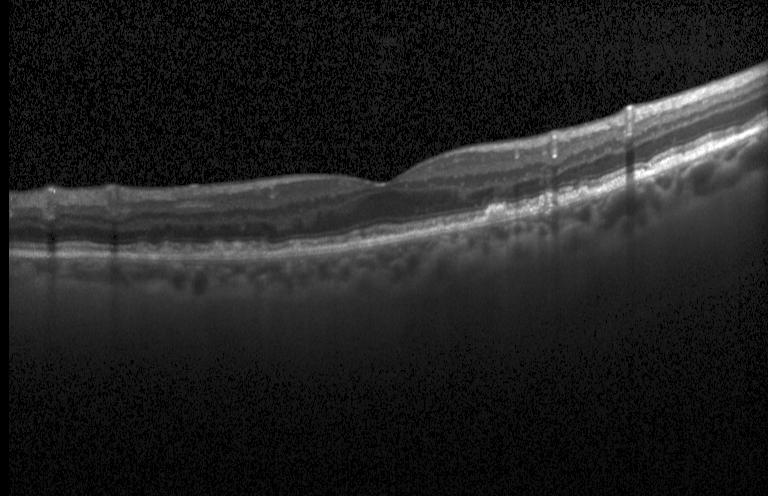 Optical coherence tomography B-scan · through the macula — Multiple drusen.